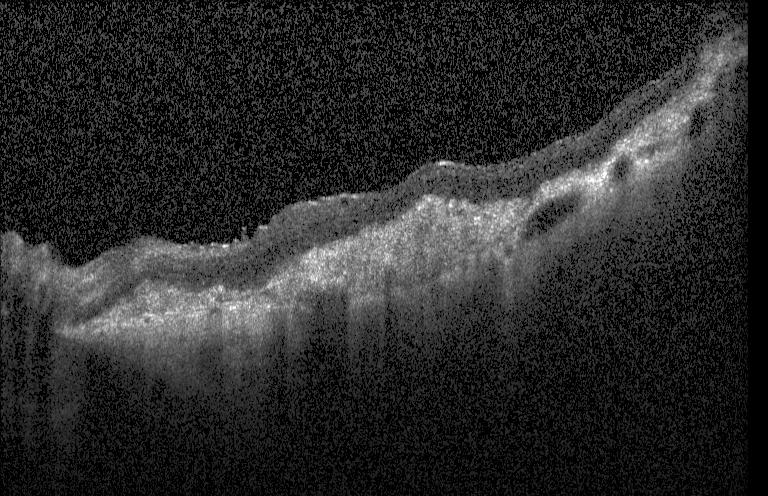
Heidelberg Spectralis OCT system · horizontal scan through the fovea · OCT line scan · spectral-domain optical coherence tomography.
This B-scan demonstrates a choroidal neovascular membrane.